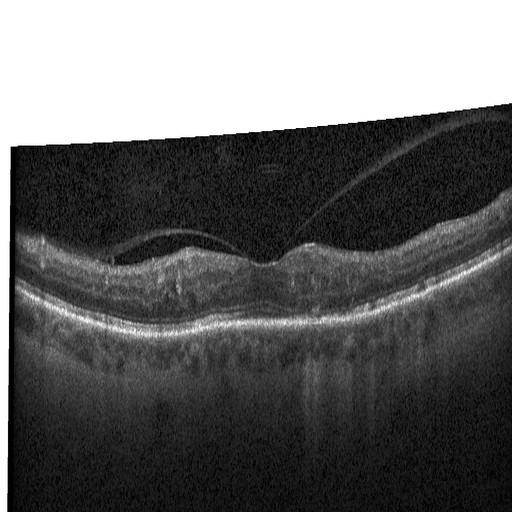
Optical coherence tomography B-scan · horizontal scan through the fovea · spectral-domain OCT
Dx: diabetic macular edema (DME).